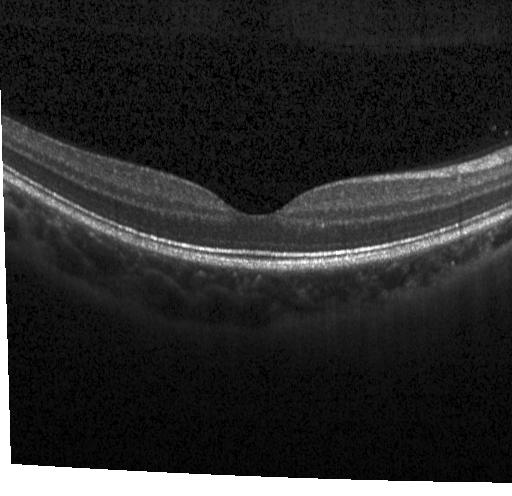

OCT B-scan. Spectral-domain optical coherence tomography. Impression: no choroidal neovascularization, diabetic macular edema, or drusen.